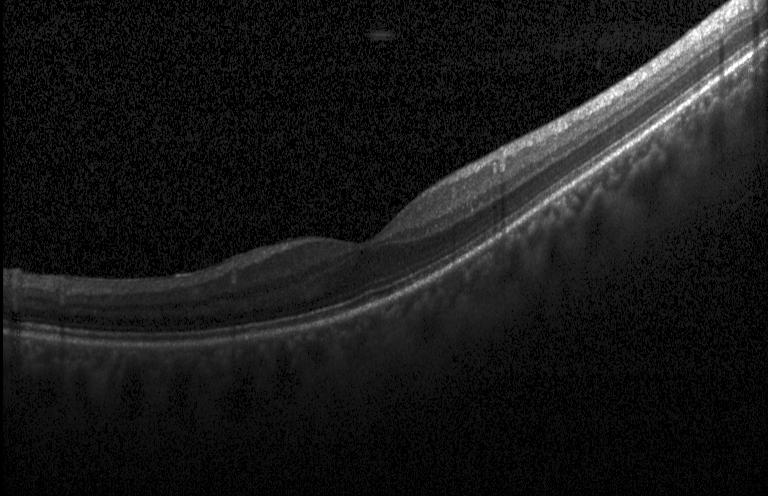
Retinal OCT cross-section showing no choroidal neovascularization, no diabetic macular edema, and no drusen.